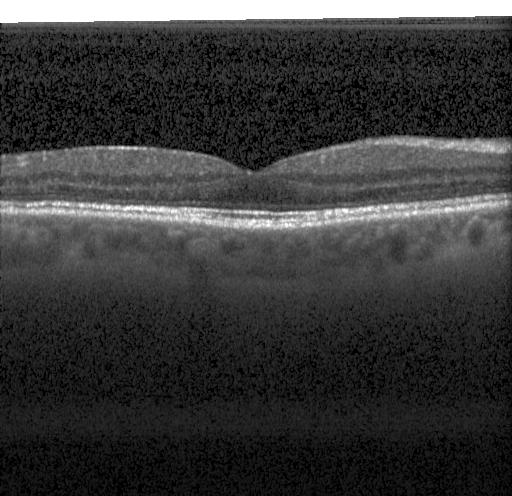 Spectral-domain optical coherence tomography, through the macula, OCT B-scan, instrument: Heidelberg Spectralis. Diagnosis: neither choroidal neovascularization, diabetic macular edema, nor drusen.